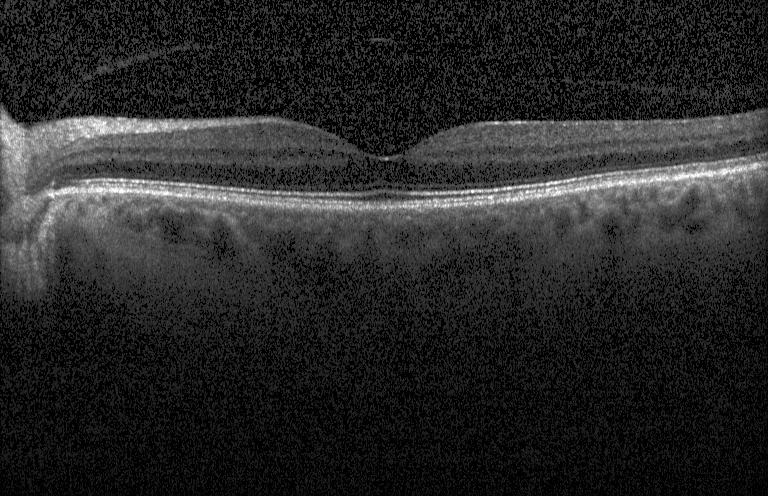 SD-OCT · OCT B-scan · Heidelberg Spectralis · through the macula — This B-scan demonstrates no CNV, DME, or drusen.